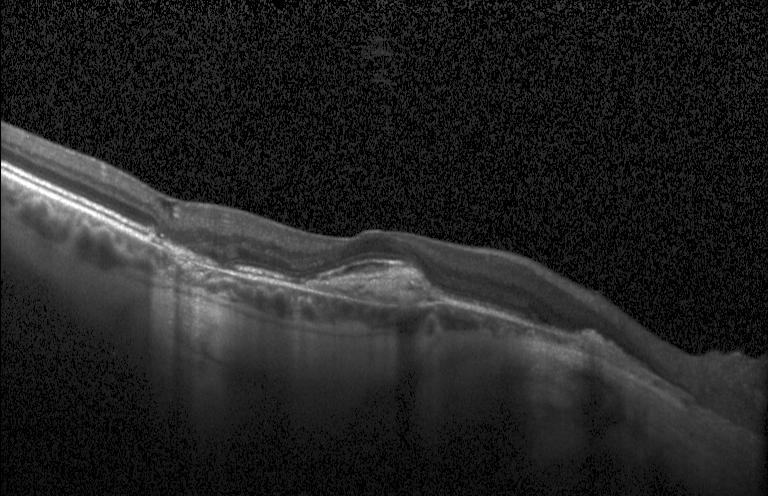 Diagnosis: a choroidal neovascular membrane.